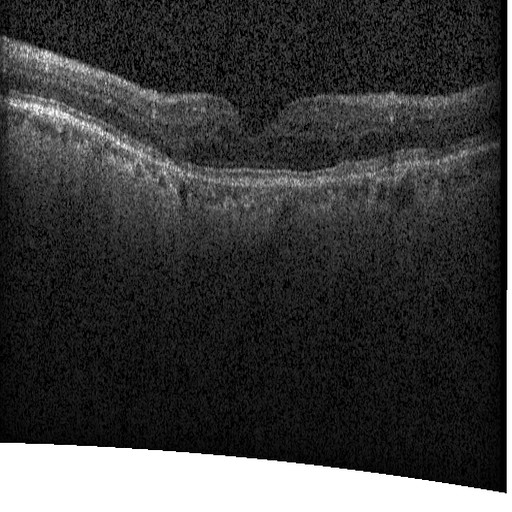

Impression: DME.